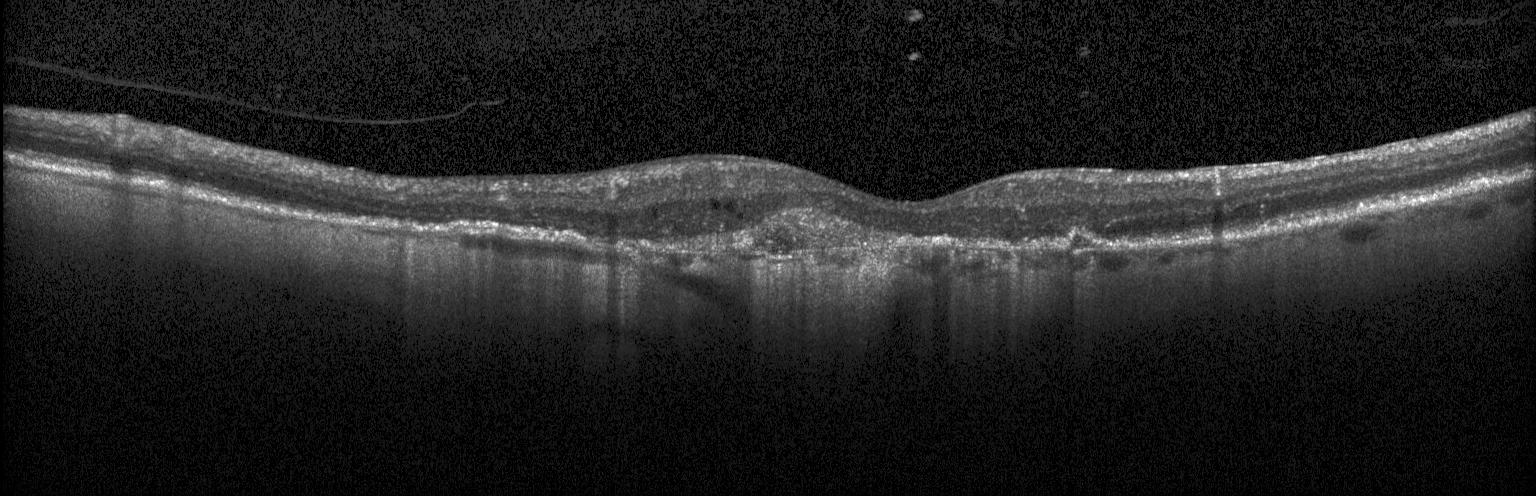

Spectral-domain OCT B-scan: a choroidal neovascular membrane.